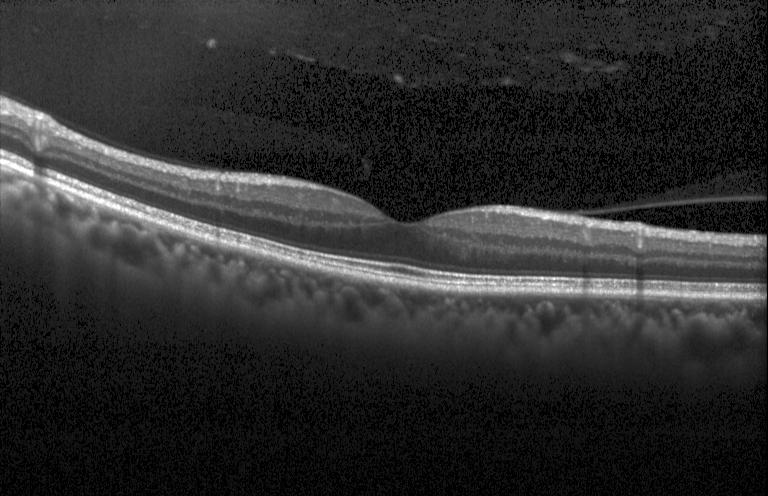
This B-scan demonstrates no choroidal neovascularization, no diabetic macular edema, and no drusen.